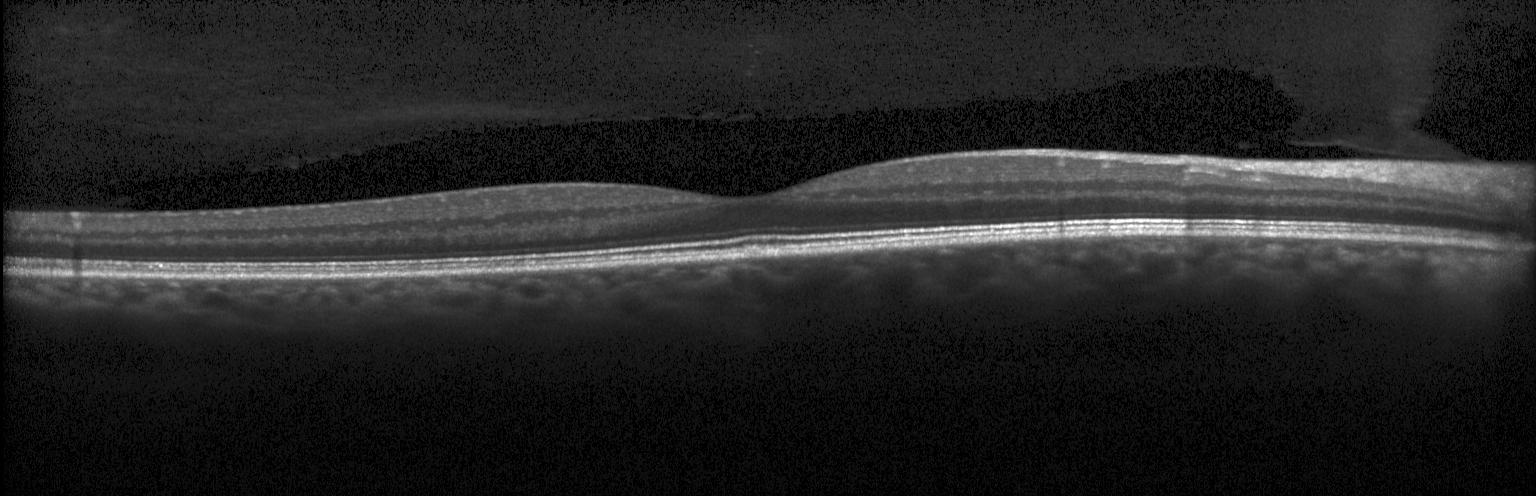 Diagnosis: neither choroidal neovascularization, diabetic macular edema, nor drusen.